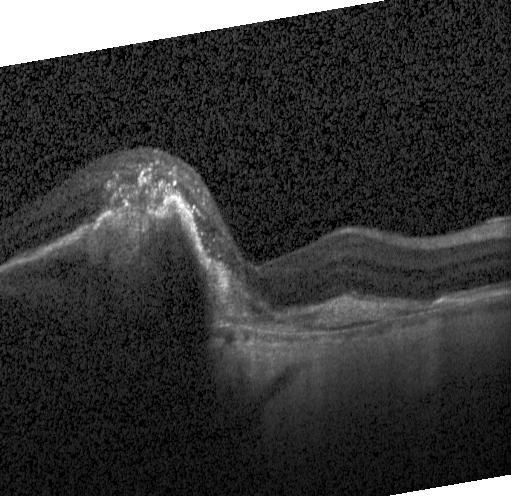 OCT line scan
The scan shows a choroidal neovascular membrane.